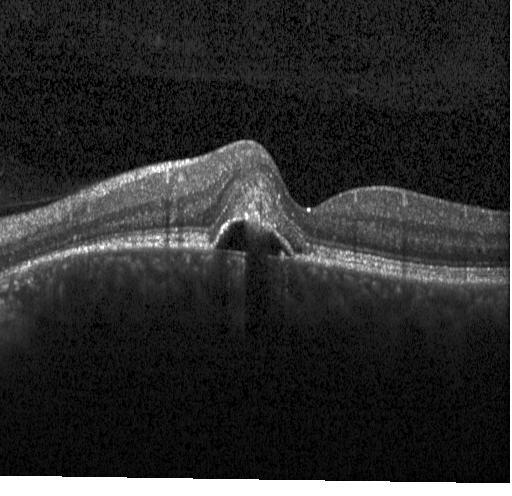
Finding: choroidal neovascularization (CNV).